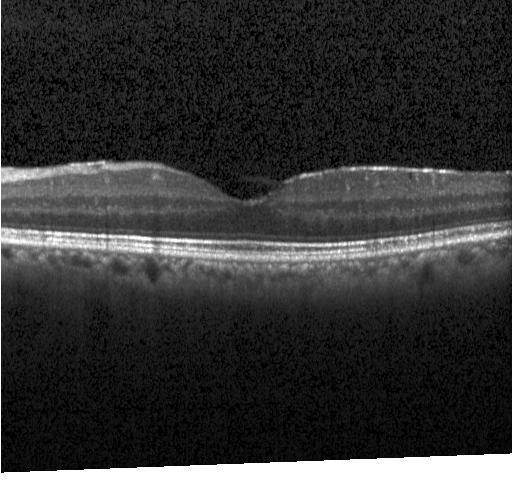 Diagnosis: no choroidal neovascularization, no diabetic macular edema, and no drusen.